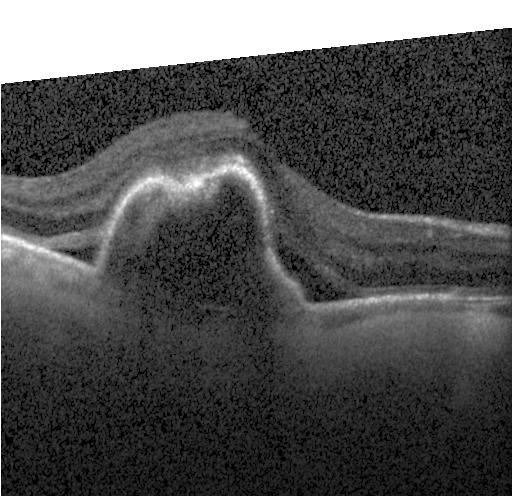

Optical coherence tomography scan
Dx: choroidal neovascularization.